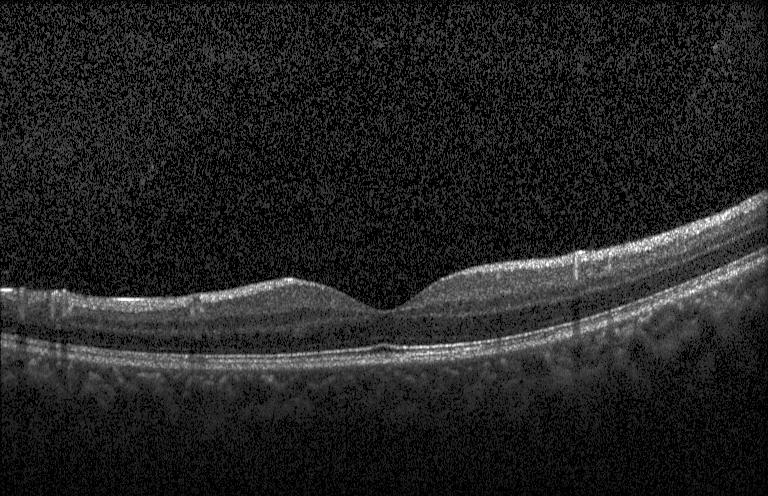

Impression: no choroidal neovascularization, no diabetic macular edema, and no drusen.